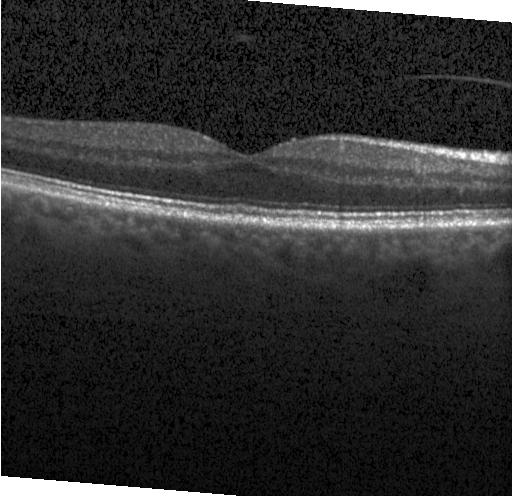 Impression: no evidence of CNV, DME, or drusen.